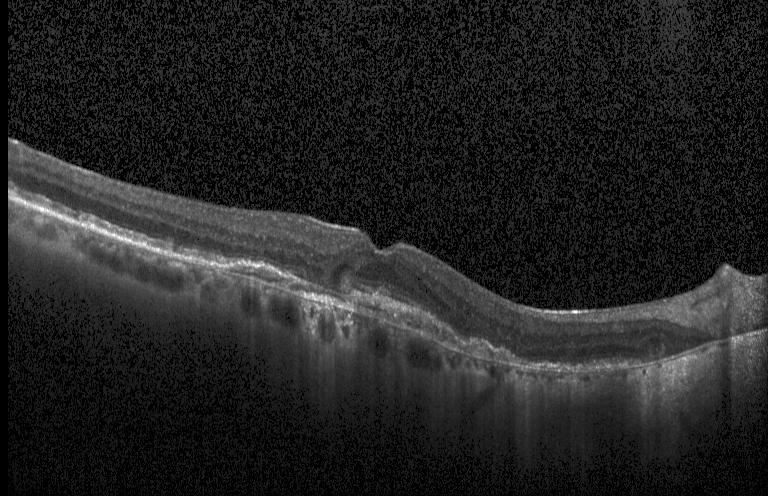

Impression: CNV.